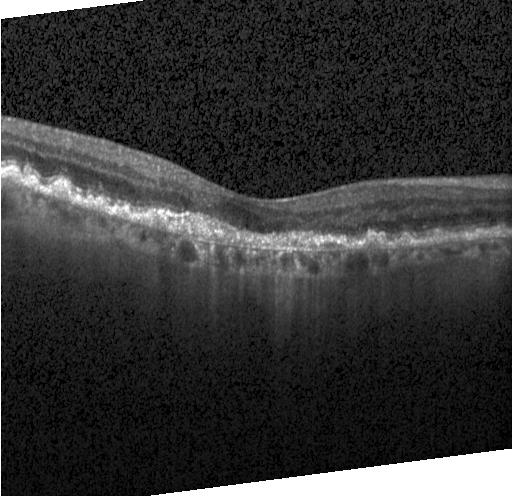
OCT line scan. Impression: choroidal neovascularization (CNV).